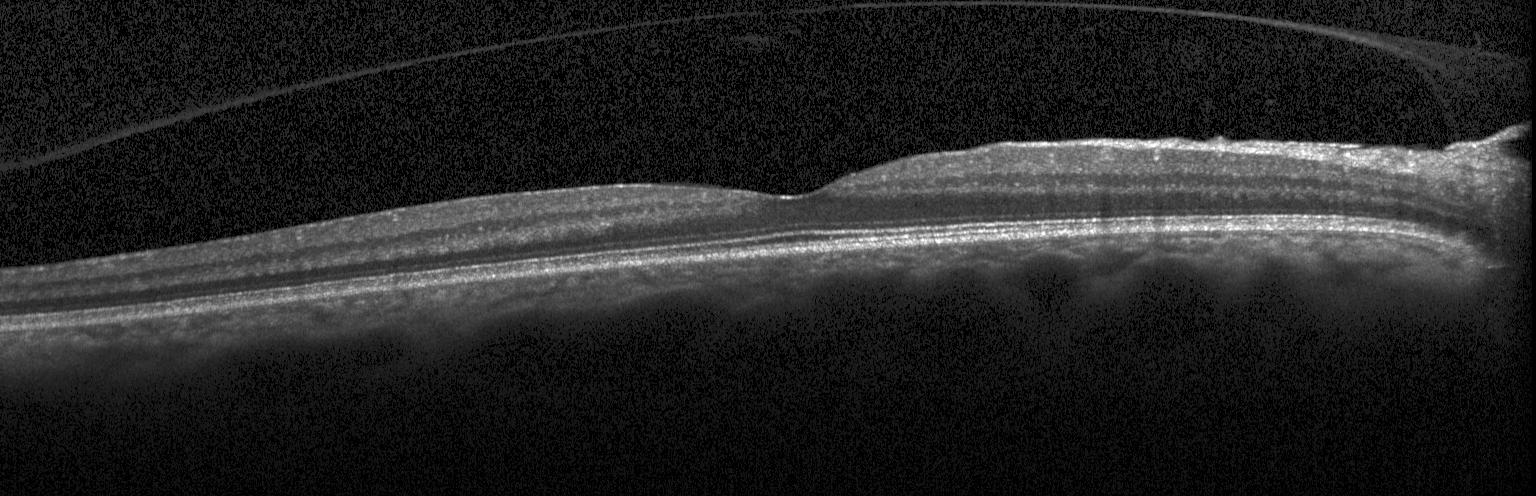
Optical coherence tomography scan · Heidelberg Spectralis.
Diagnosis: no choroidal neovascularization, no diabetic macular edema, and no drusen.